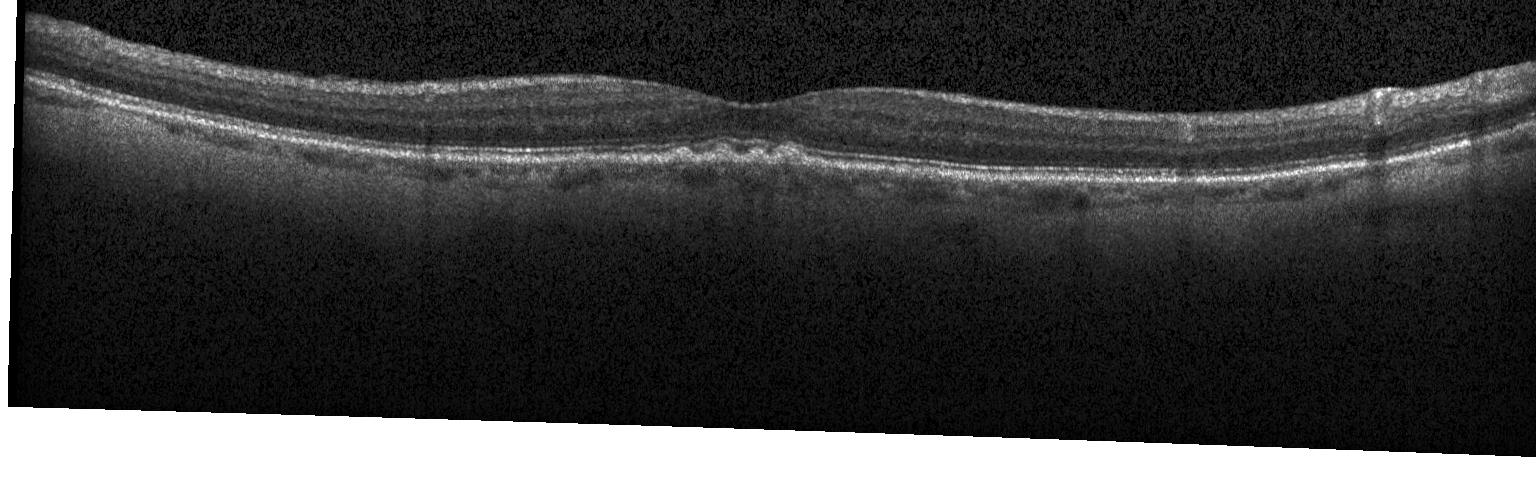

Macular OCT demonstrating multiple drusen.